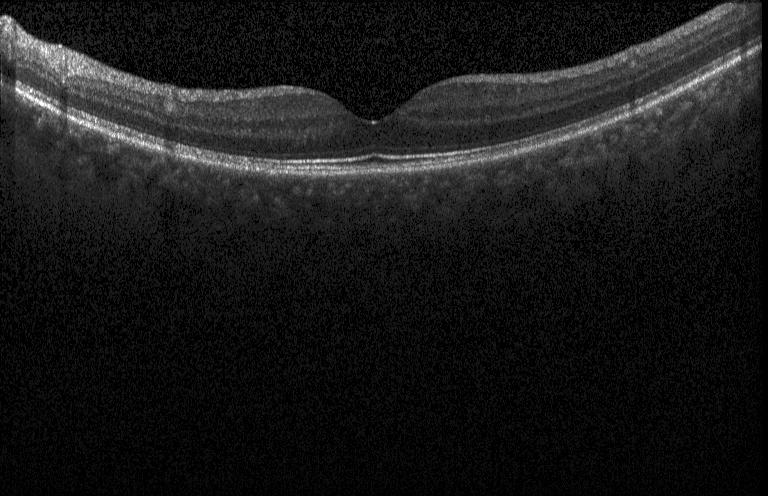

Retinal OCT B-scan. Acquired on a Heidelberg Spectralis — Dx: neither CNV, DME, nor drusen.